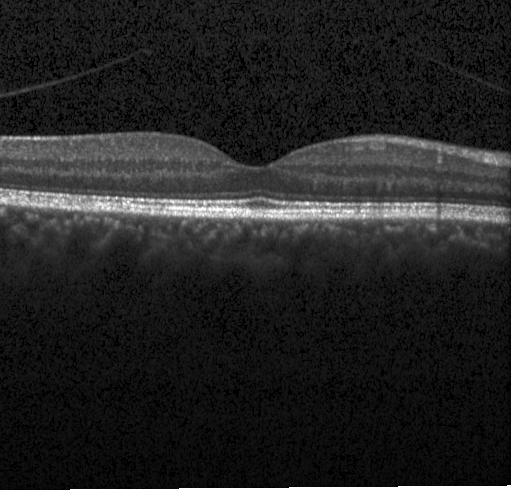

Macular scan; SD-OCT; optical coherence tomography scan — OCT finding: no evidence of CNV, DME, or drusen.